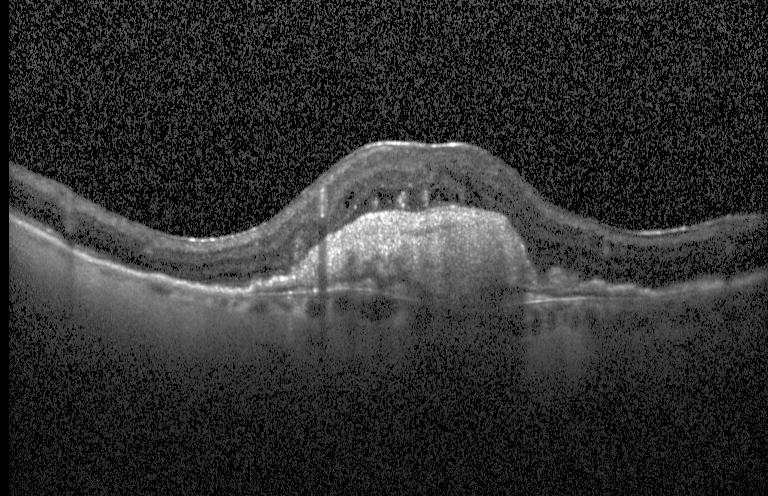

Optical coherence tomography scan
Diagnosis: a choroidal neovascular membrane.